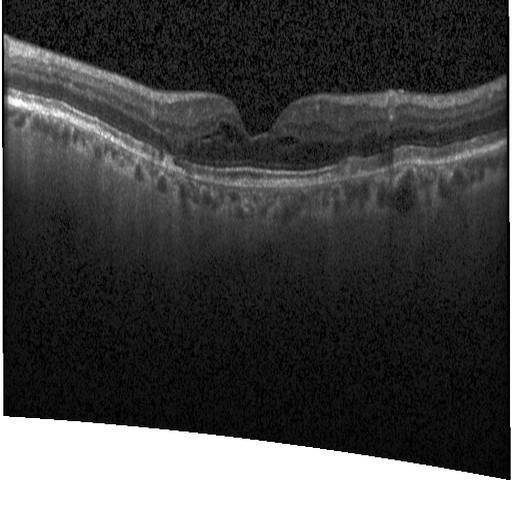 Finding: DME.